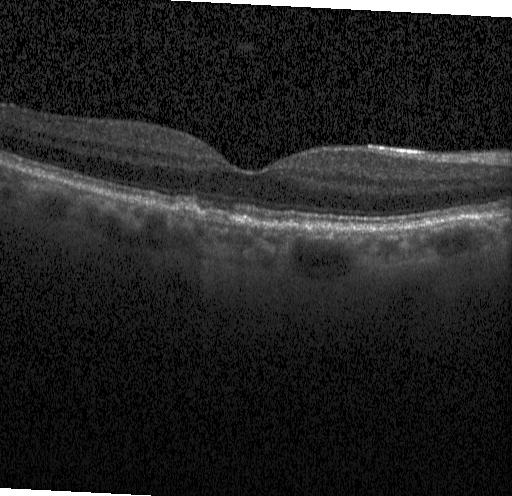
Spectral-domain OCT B-scan: drusen.